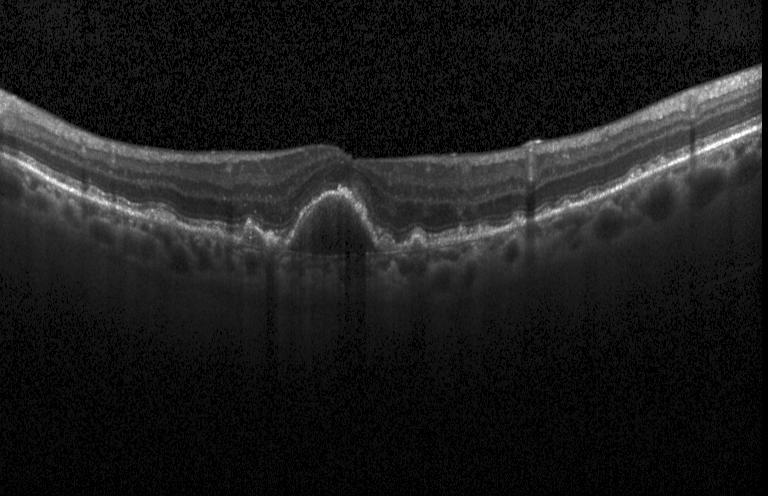

OCT B-scan, fovea-centered. A choroidal neovascular membrane.